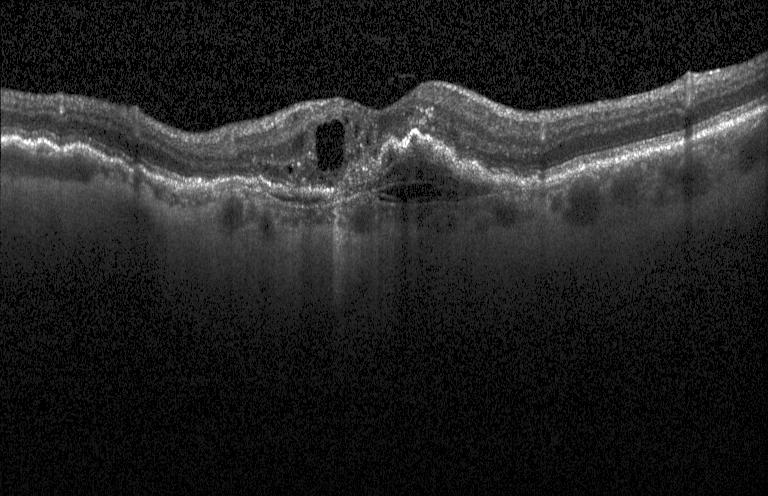

Through the macula · SD-OCT · OCT line scan
Diagnosis: a choroidal neovascular membrane.